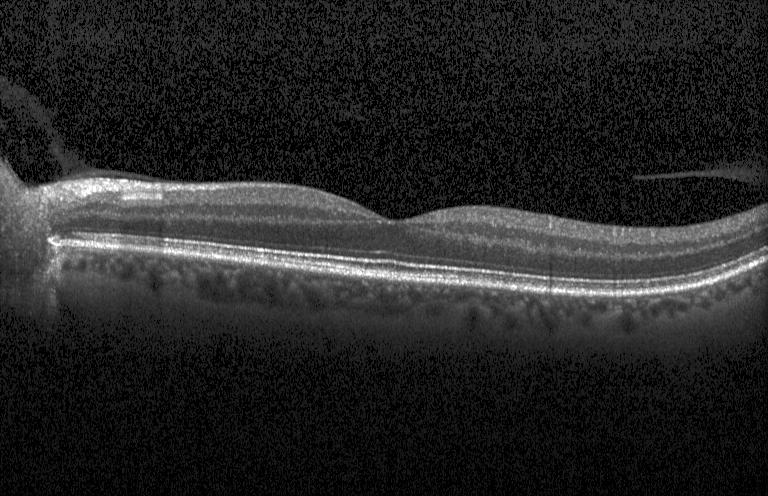
OCT line scan, Heidelberg Spectralis OCT system, fovea-centered, SD-OCT — Macular OCT: neither CNV, DME, nor drusen.